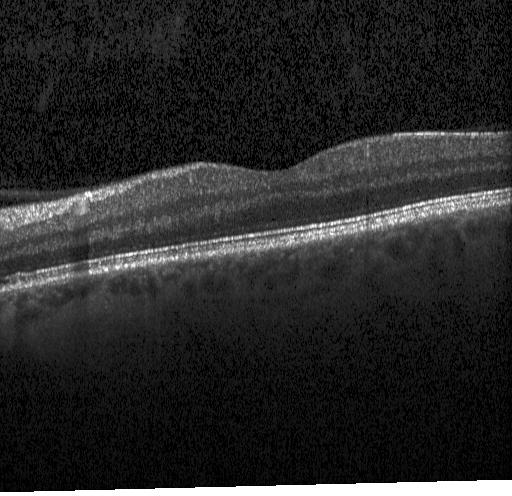 Spectral-domain OCT B-scan: neither choroidal neovascularization, diabetic macular edema, nor drusen.